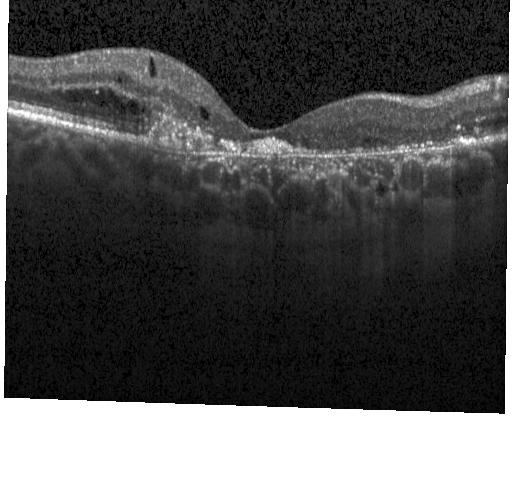
OCT B-scan. This B-scan demonstrates a choroidal neovascular membrane.